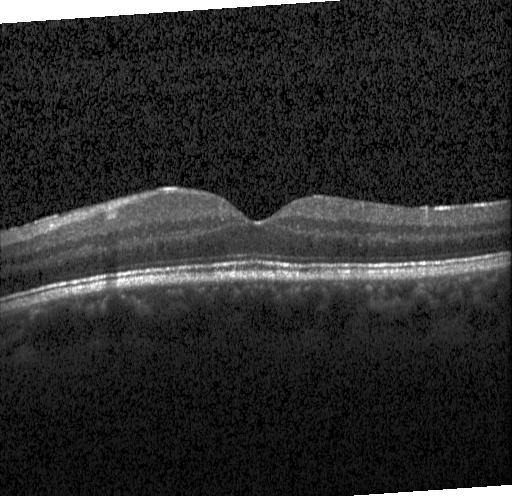
Diagnosis: no evidence of choroidal neovascularization, diabetic macular edema, or drusen.